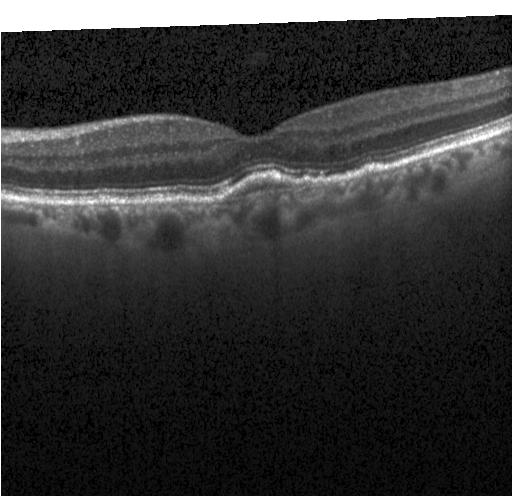 Impression: a choroidal neovascular membrane.